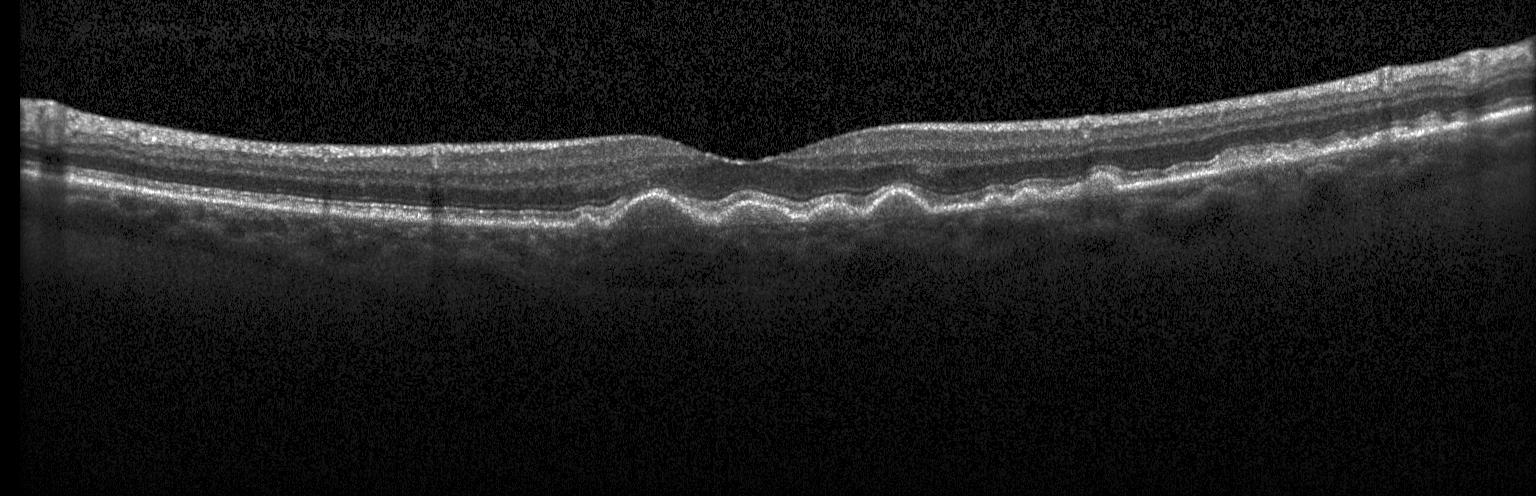 Optical coherence tomography B-scan · through the macula · Heidelberg Spectralis · spectral-domain optical coherence tomography.
Impression: drusen.